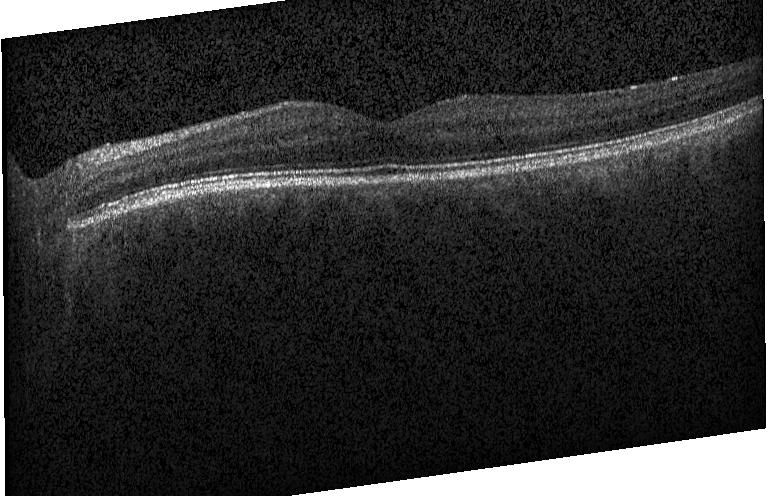 OCT line scan · spectral-domain OCT.
Finding: no evidence of choroidal neovascularization, diabetic macular edema, or drusen.